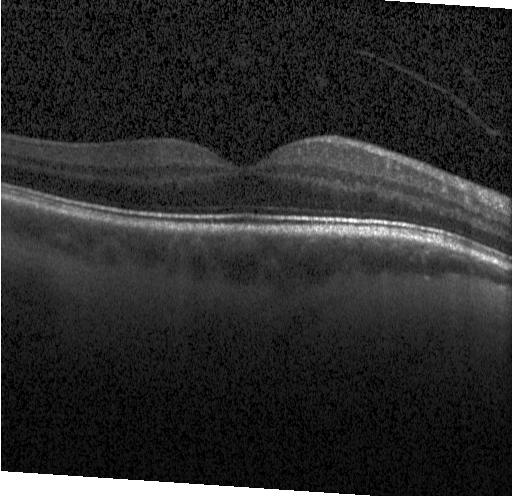 OCT finding: neither choroidal neovascularization, diabetic macular edema, nor drusen.